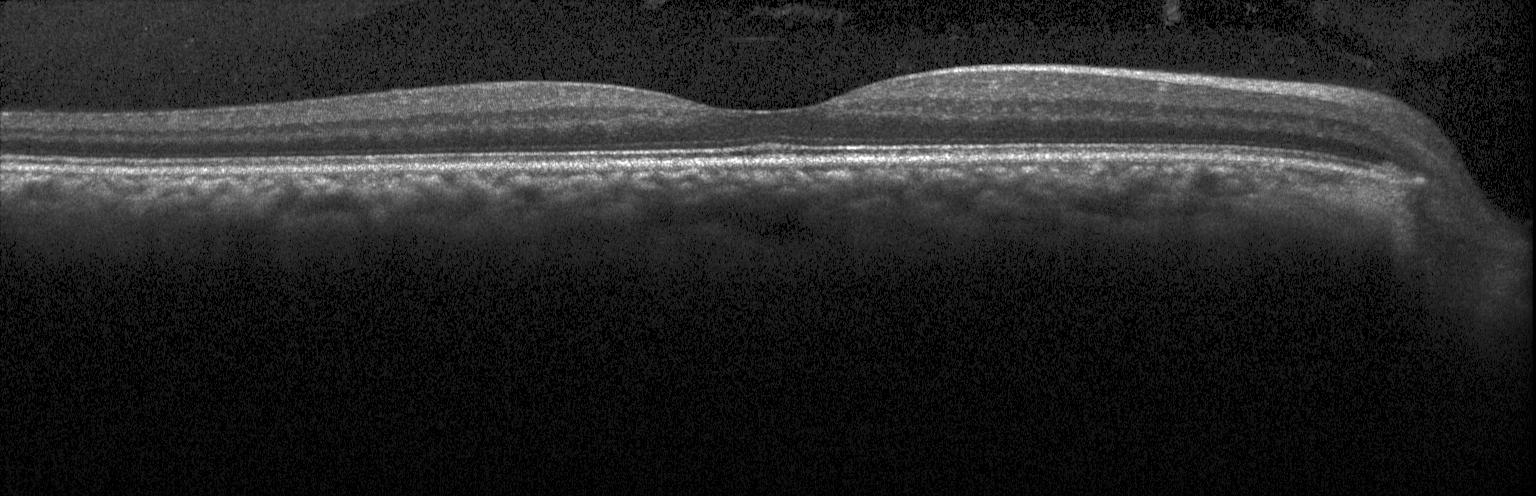

OCT scan showing no choroidal neovascularization, no diabetic macular edema, and no drusen.